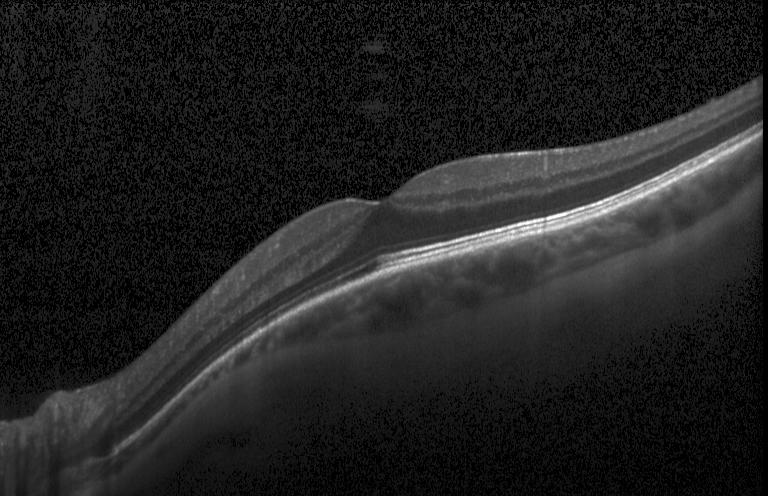

Heidelberg Spectralis, OCT line scan, spectral-domain OCT, fovea-centered — Assessment: no choroidal neovascularization, no diabetic macular edema, and no drusen.